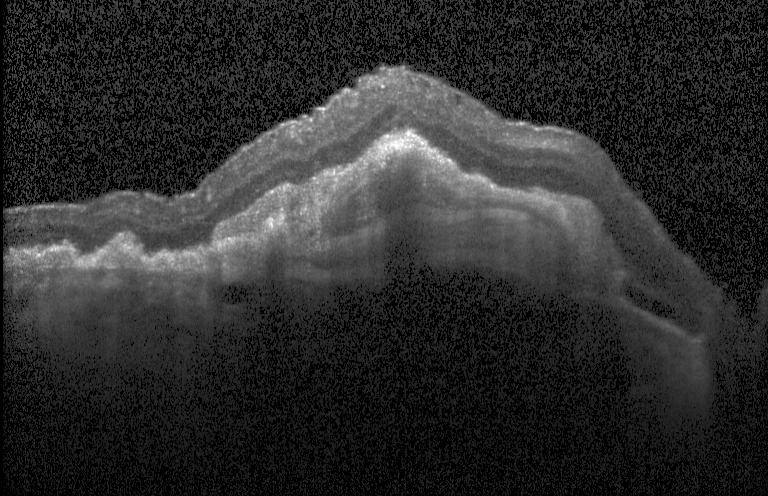
OCT scan showing CNV.